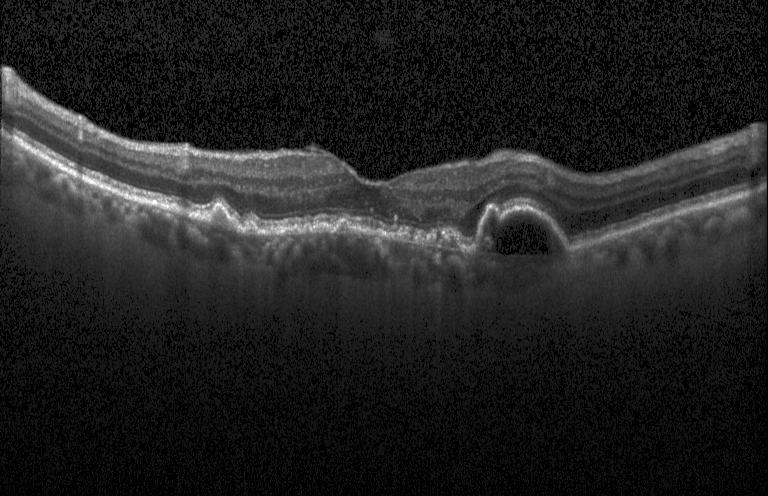 OCT scan showing choroidal neovascularization (CNV).